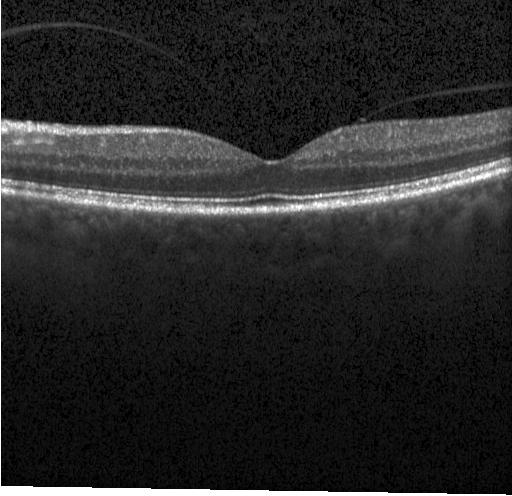 OCT B-scan showing neither choroidal neovascularization, diabetic macular edema, nor drusen.